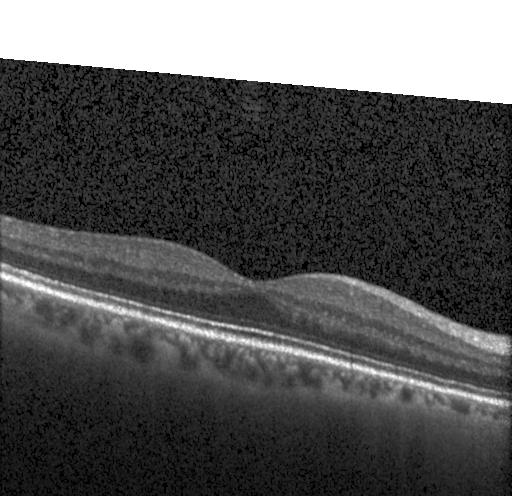 Retinal OCT cross-section. Heidelberg Spectralis. SD-OCT. Diagnosis: no evidence of CNV, DME, or drusen.